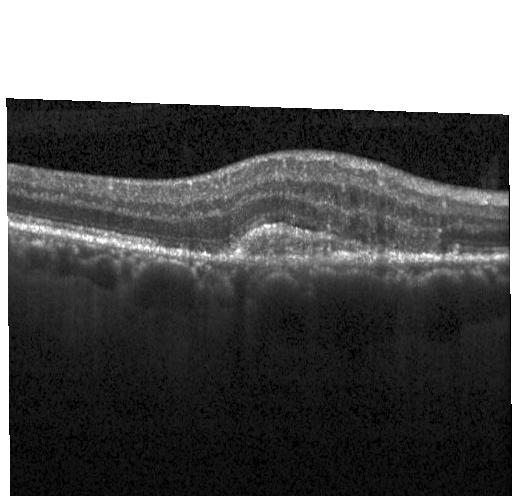 SD-OCT. Retinal OCT B-scan
Impression: a choroidal neovascular membrane.